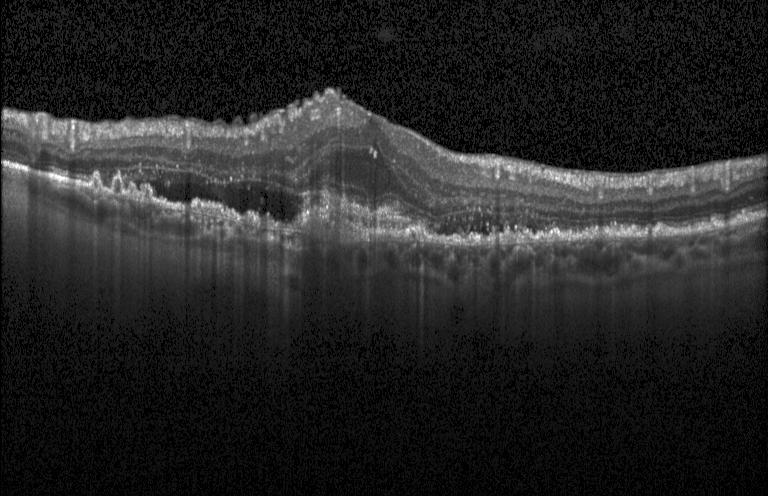

OCT finding: choroidal neovascularization.